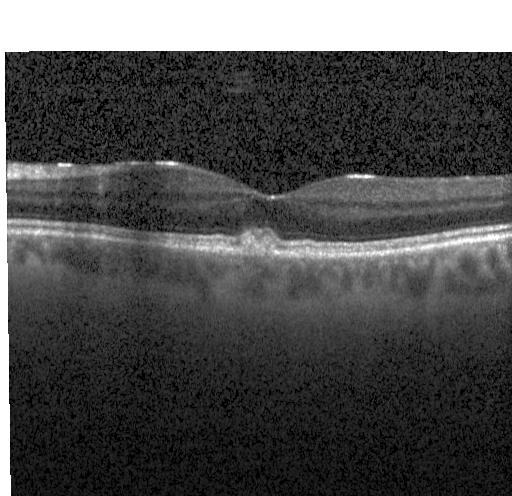
Spectral-domain OCT, horizontal scan through the fovea, Heidelberg Spectralis, OCT B-scan.
Impression: sub-RPE drusenoid deposits.